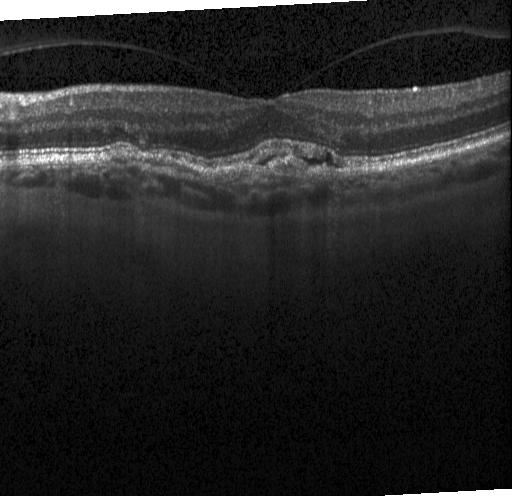 Heidelberg Spectralis; retinal OCT B-scan; macular scan
Macular OCT: choroidal neovascularization.